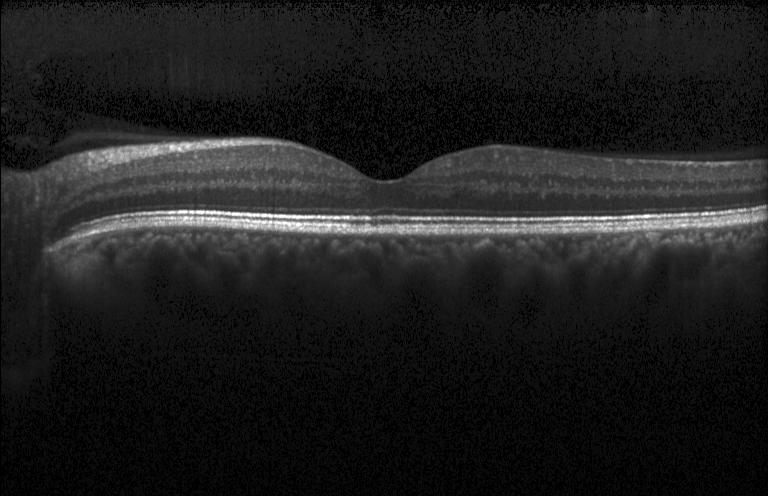
Spectral-domain OCT, horizontal scan through the fovea, OCT line scan — This B-scan demonstrates neither CNV, DME, nor drusen.